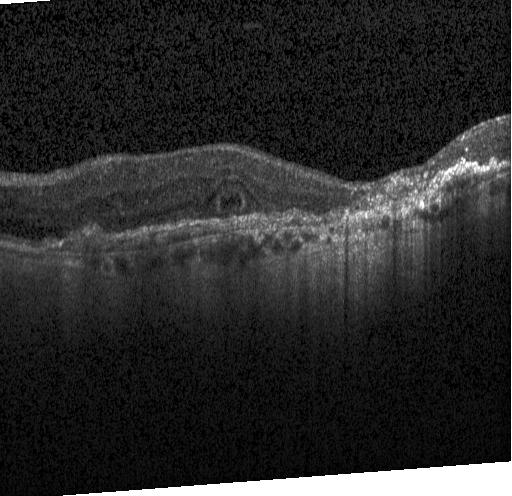

SD-OCT; optical coherence tomography B-scan; through the macula
Macular OCT: a choroidal neovascular membrane.